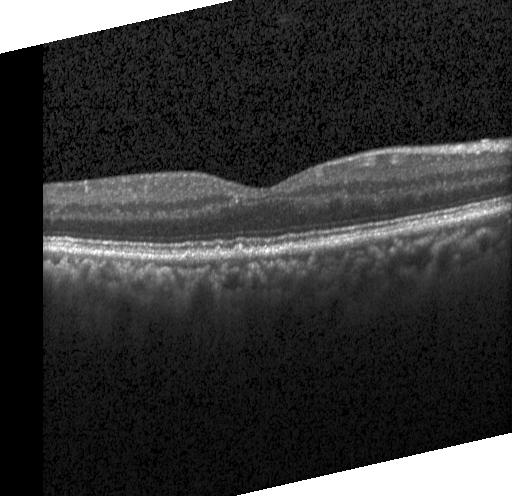
Retinal OCT cross-section showing multiple drusen.